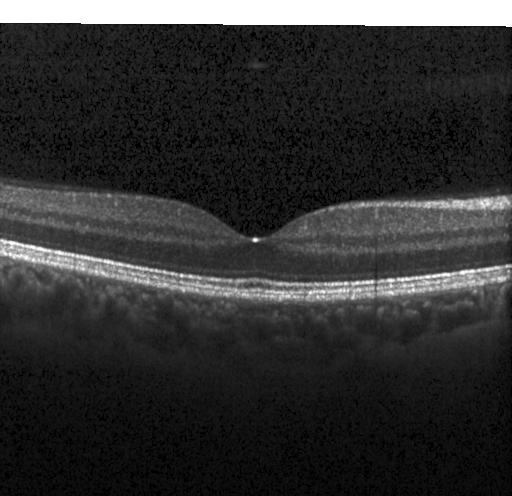
OCT B-scan, acquired on a Heidelberg Spectralis, macular scan, spectral-domain OCT. No choroidal neovascularization, no diabetic macular edema, and no drusen.